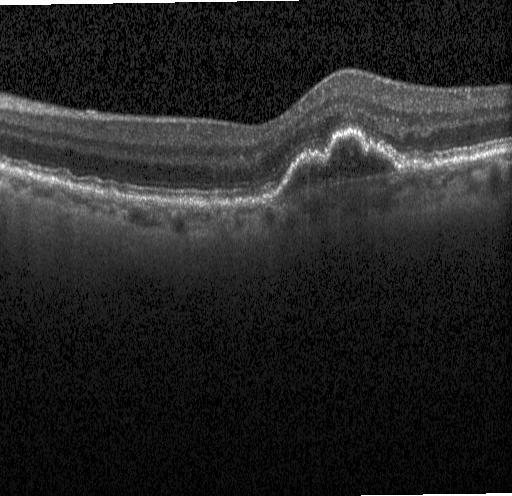 Retinal OCT B-scan · acquired on a Heidelberg Spectralis.
Diagnosis: a choroidal neovascular membrane.